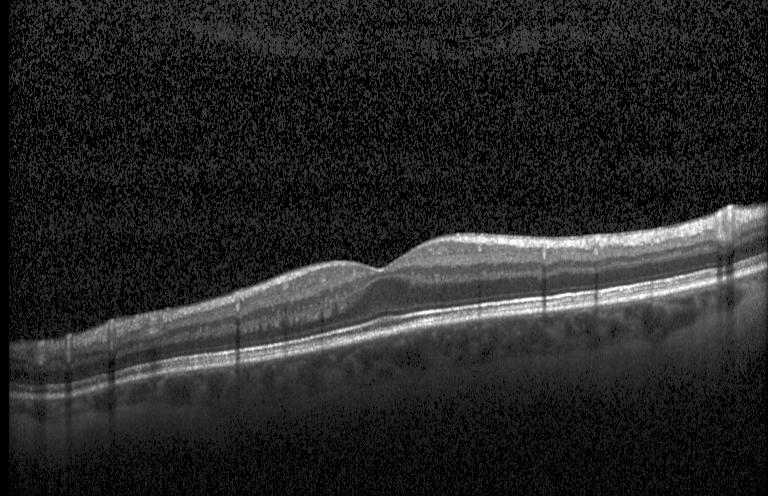
Finding: neither choroidal neovascularization, diabetic macular edema, nor drusen.